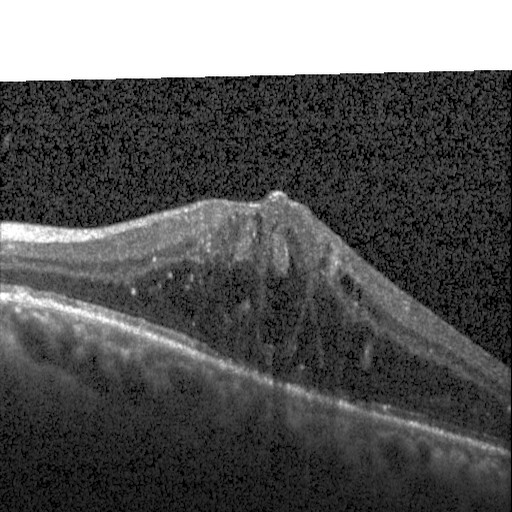 This B-scan demonstrates diabetic macular edema (DME).